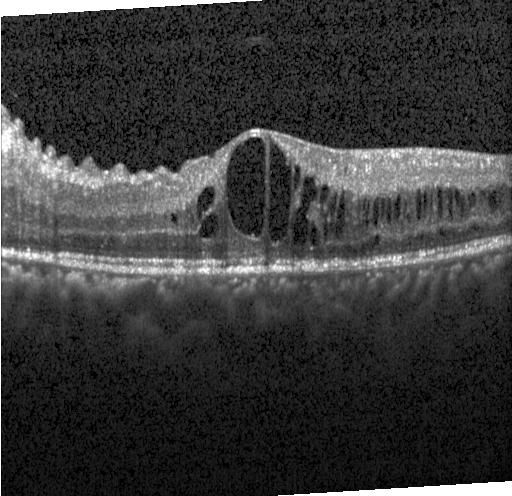

This B-scan demonstrates diabetic macular edema.